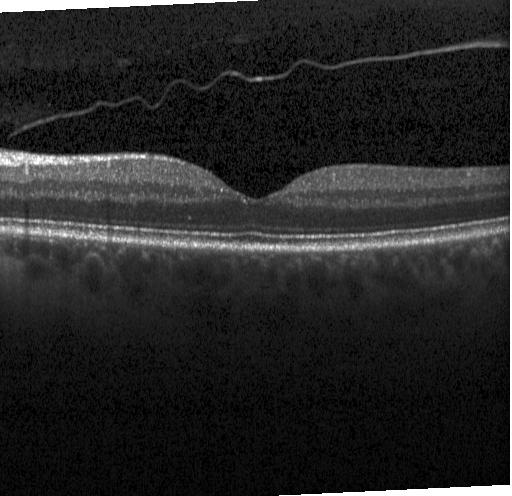

Macular OCT: no CNV, DME, or drusen.